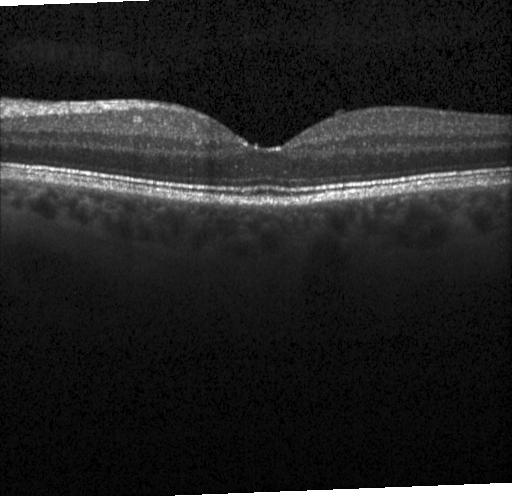
Retinal OCT B-scan. Finding: no choroidal neovascularization, no diabetic macular edema, and no drusen.